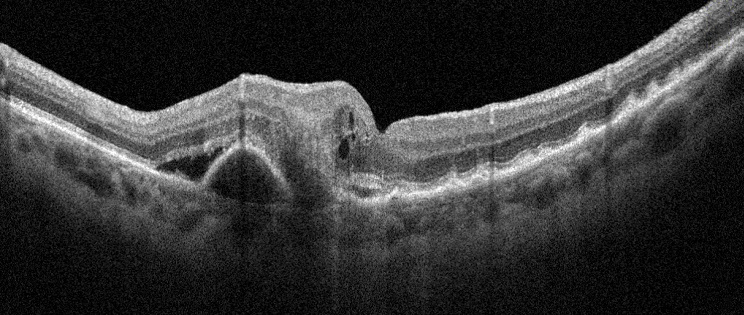

OCT B-scan, instrument: Optovue Avanti RTVue XR, macular scan
Finding: AMD.